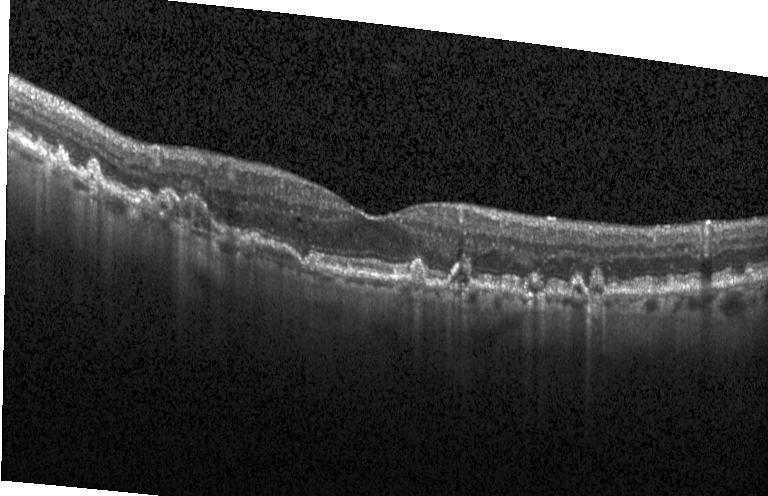

Spectral-domain optical coherence tomography, fovea-centered, OCT line scan, Heidelberg Spectralis — Finding: choroidal neovascularization (CNV).